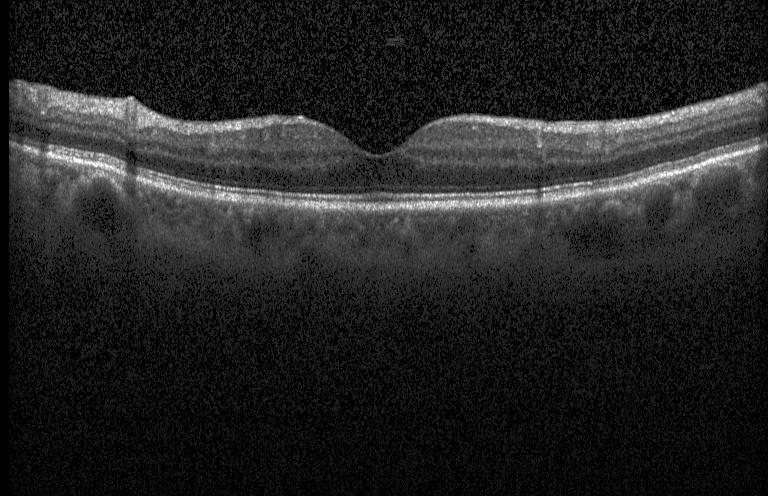 Spectral-domain optical coherence tomography. Fovea-centered. Optical coherence tomography scan. Heidelberg Spectralis OCT system
The scan shows no CNV, no DME, and no drusen.